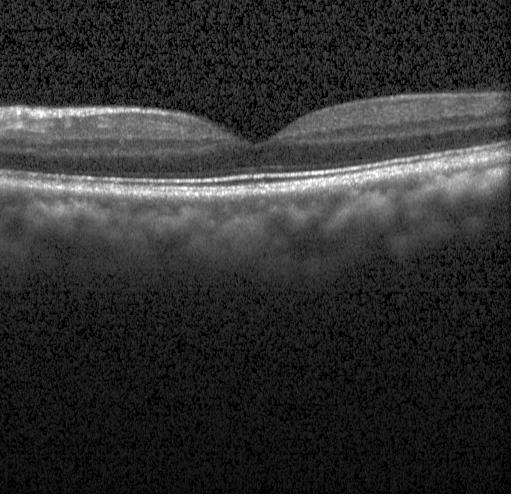

Macular OCT: no choroidal neovascularization, diabetic macular edema, or drusen.